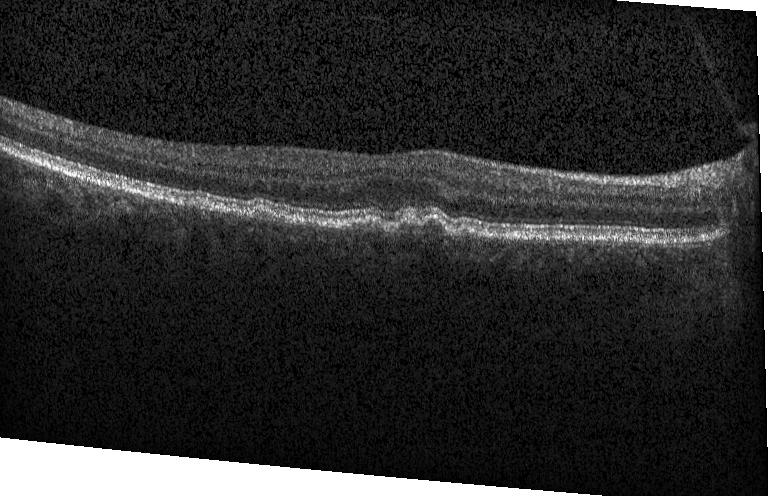

Optical coherence tomography scan
Diagnosis: drusen.